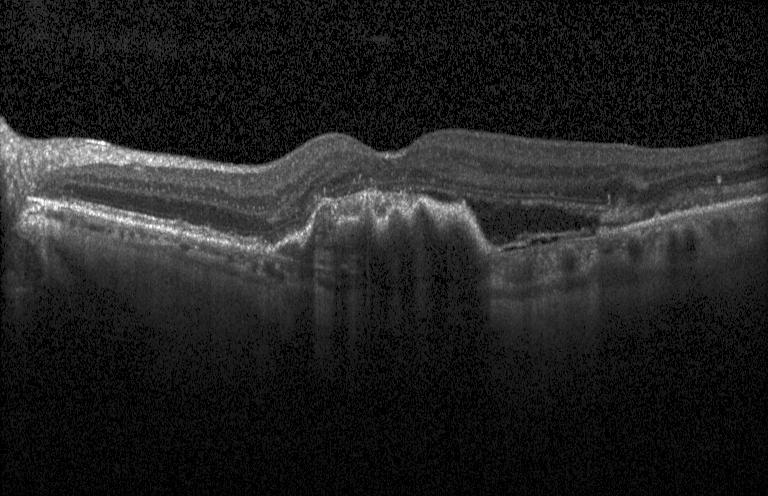

Retinal OCT B-scan. Acquired on a Heidelberg Spectralis — The scan shows choroidal neovascularization (CNV).